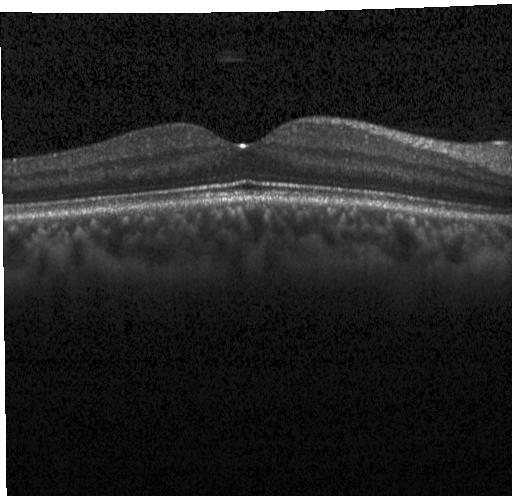 Retinal OCT B-scan. Diagnosis: no evidence of CNV, DME, or drusen.